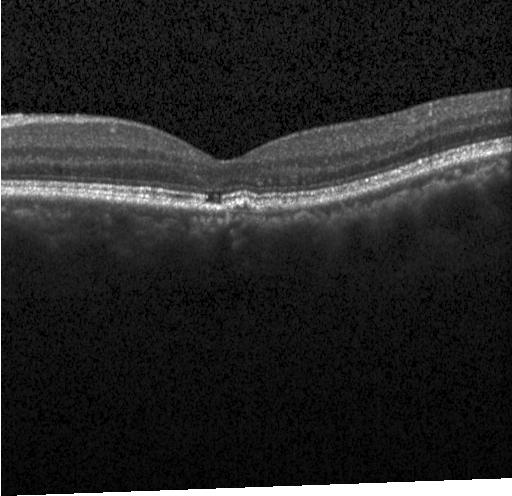

Horizontal scan through the fovea · retinal OCT cross-section · acquired on a Heidelberg Spectralis
OCT finding: multiple drusen.